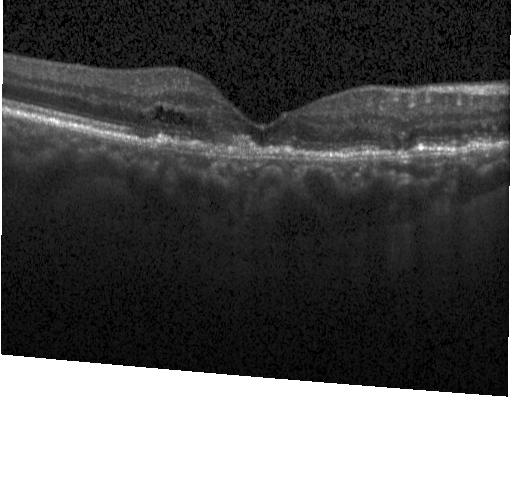

This B-scan demonstrates CNV.